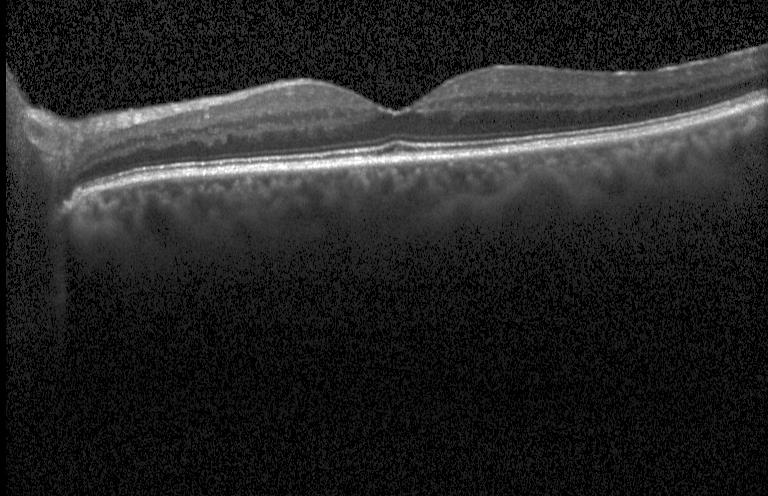 Retinal OCT B-scan
OCT finding: no choroidal neovascularization, diabetic macular edema, or drusen.